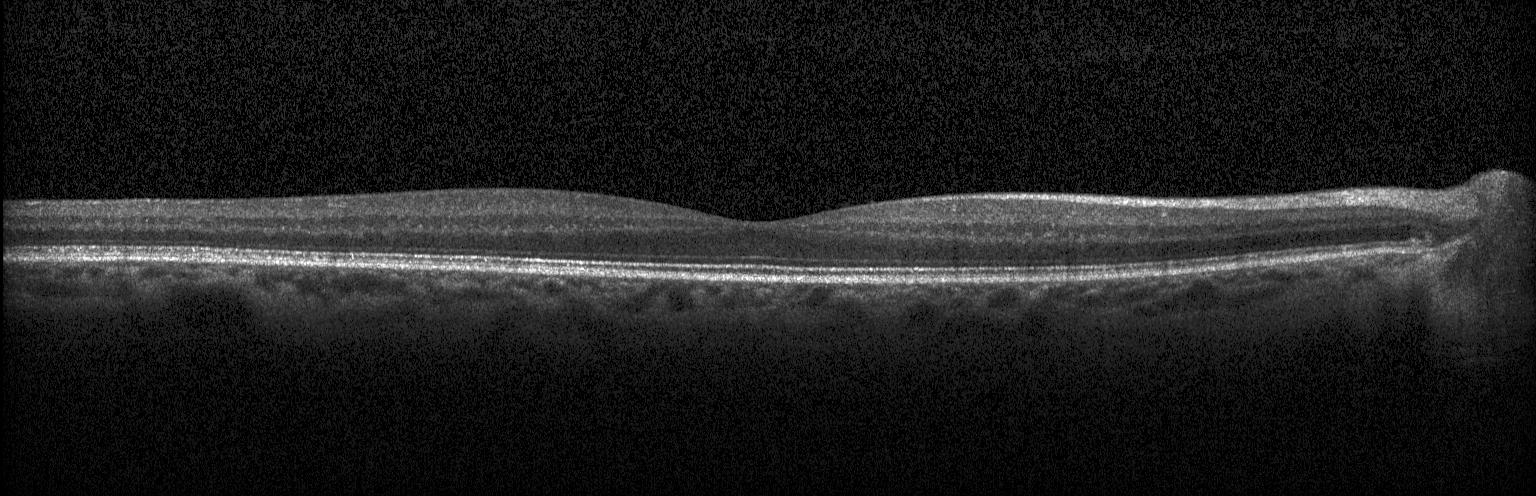
Retinal OCT cross-section. This B-scan demonstrates no CNV, DME, or drusen.